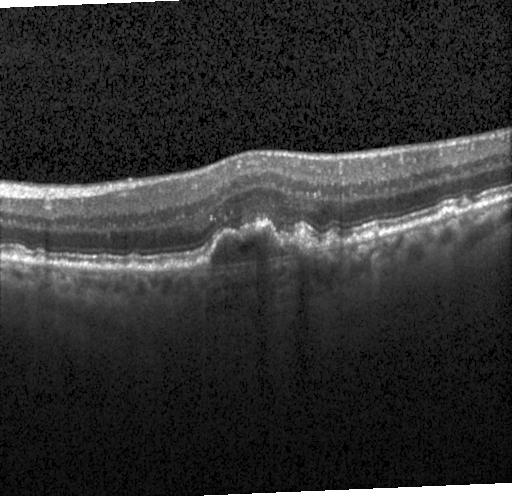 SD-OCT. Fovea-centered. OCT B-scan. Heidelberg Spectralis. Diagnosis: a choroidal neovascular membrane.